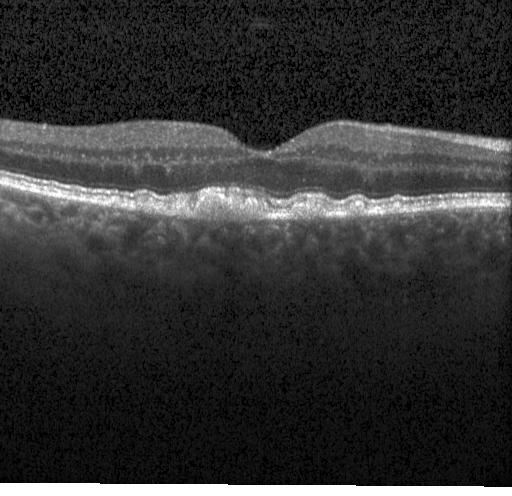 Assessment: drusen.